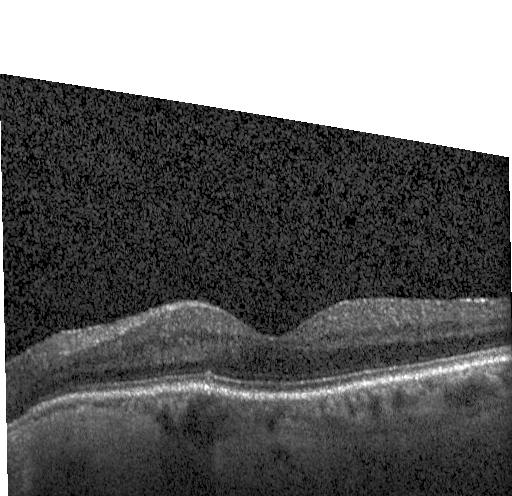
Centered on the fovea. Instrument: Heidelberg Spectralis. Retinal OCT B-scan. SD-OCT — Multiple drusen.